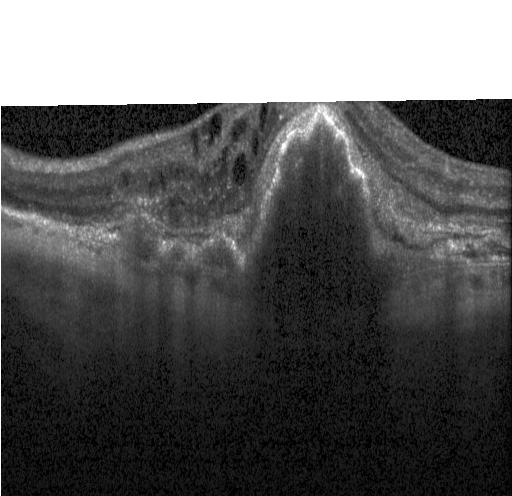

OCT scan showing CNV.